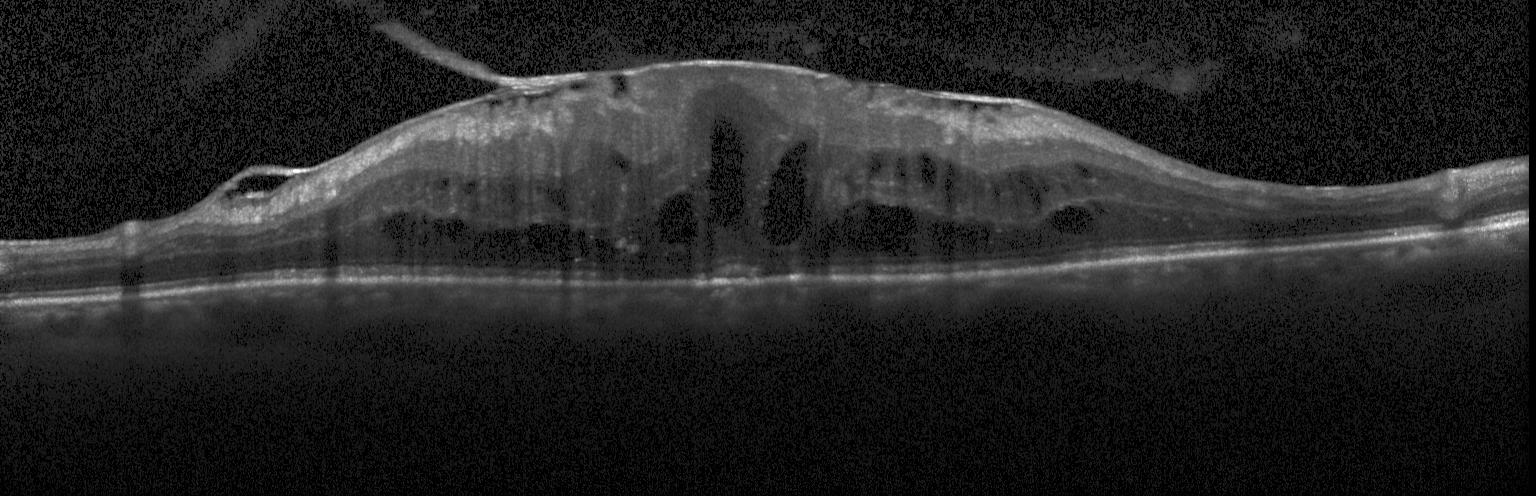
OCT line scan, centered on the fovea
Diagnosis: DME.